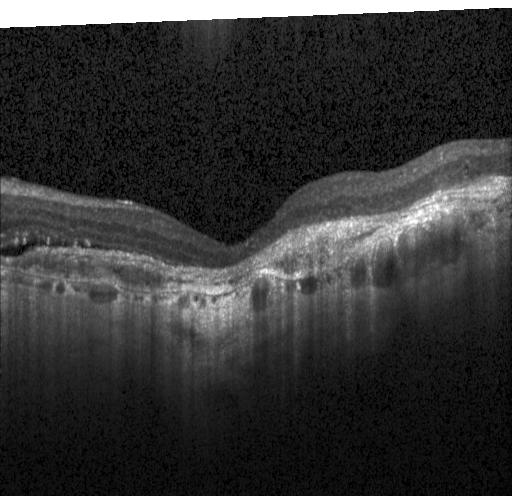 Centered on the fovea. Spectral-domain optical coherence tomography. Acquired on a Heidelberg Spectralis. Optical coherence tomography B-scan — Assessment: choroidal neovascularization (CNV).